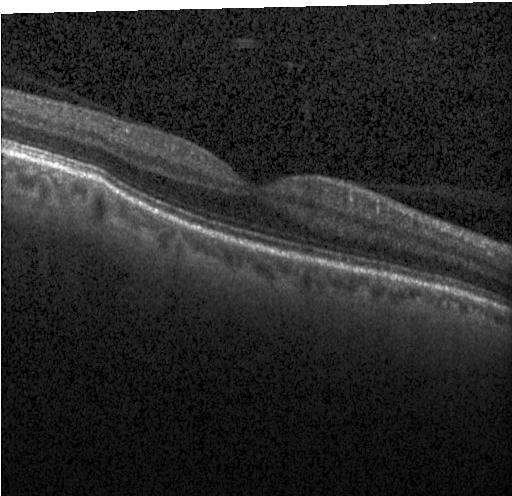 Spectral-domain OCT · centered on the fovea · optical coherence tomography B-scan · acquired on a Heidelberg Spectralis. Finding: neither choroidal neovascularization, diabetic macular edema, nor drusen.